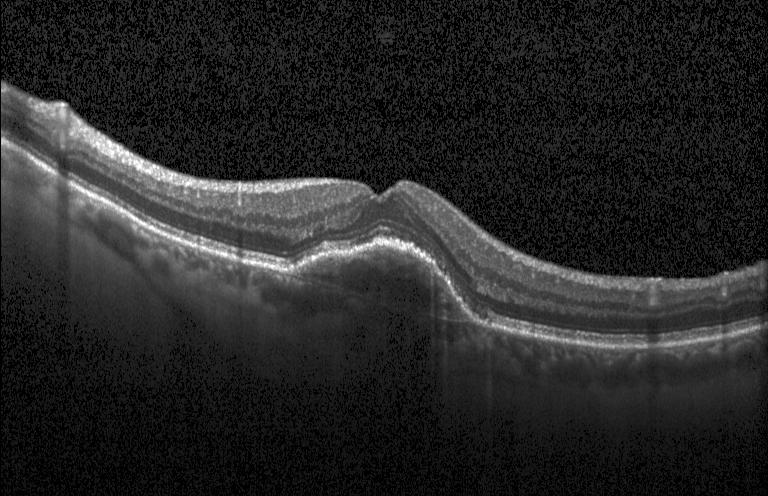 OCT finding: a choroidal neovascular membrane.